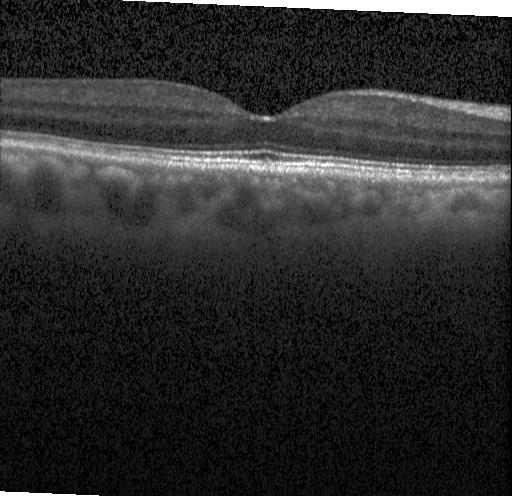 OCT B-scan; spectral-domain OCT; acquired on a Heidelberg Spectralis — Diagnosis: no evidence of choroidal neovascularization, diabetic macular edema, or drusen.